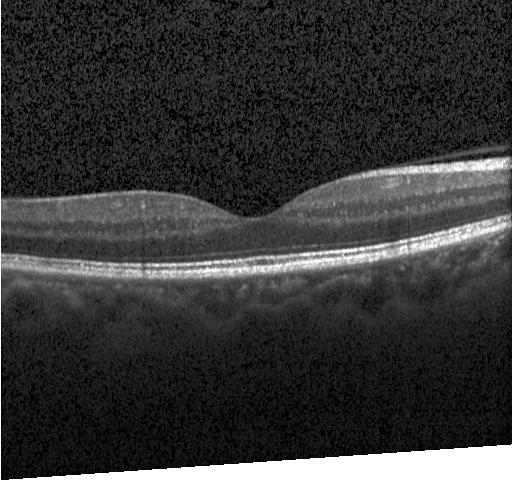 OCT B-scan. Through the macula. Instrument: Heidelberg Spectralis. Diagnosis: no evidence of CNV, DME, or drusen.